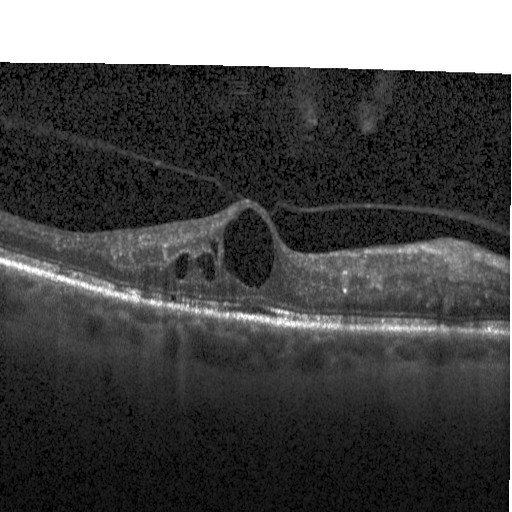

Impression: diabetic macular edema.